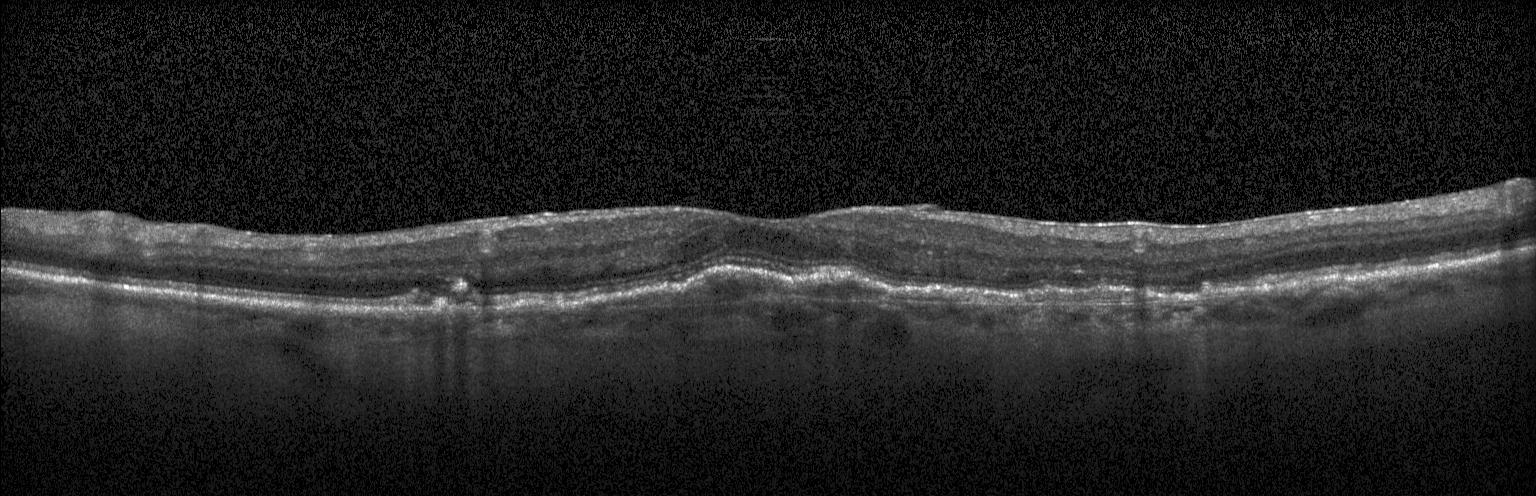

SD-OCT. OCT line scan. Macular scan. Instrument: Heidelberg Spectralis
OCT finding: a choroidal neovascular membrane.